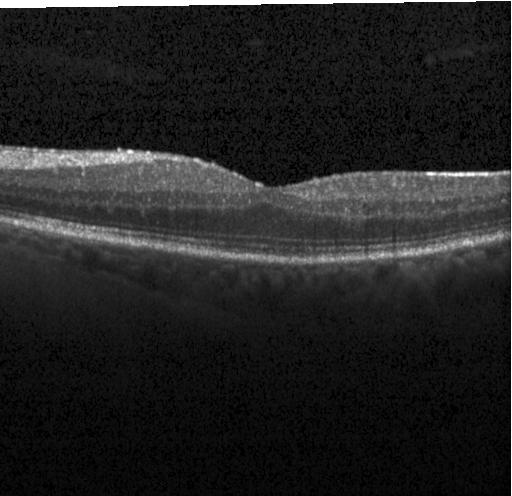

Spectral-domain optical coherence tomography · acquired on a Heidelberg Spectralis · optical coherence tomography scan · horizontal scan through the fovea
Macular OCT: no evidence of CNV, DME, or drusen.